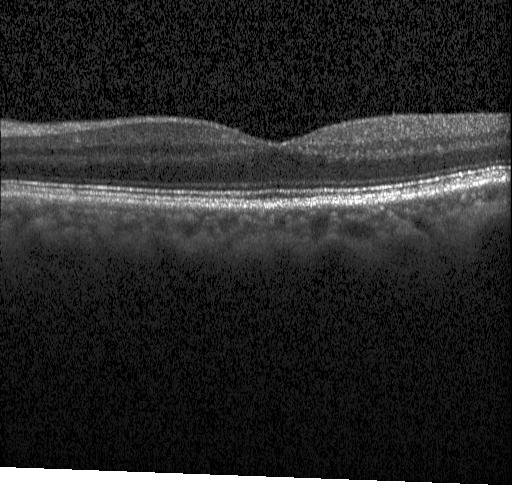

The scan shows no evidence of choroidal neovascularization, diabetic macular edema, or drusen.